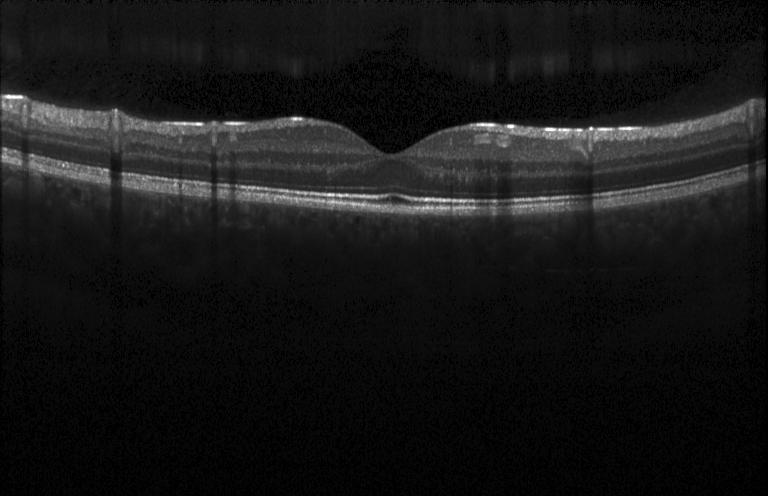

Retinal OCT B-scan.
No choroidal neovascularization, diabetic macular edema, or drusen.